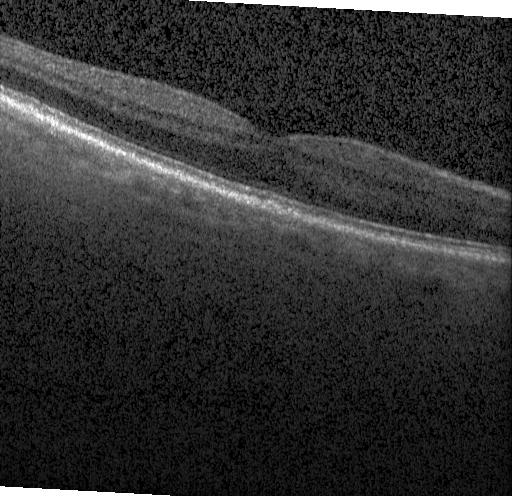 Retinal OCT cross-section. Assessment: no evidence of choroidal neovascularization, diabetic macular edema, or drusen.